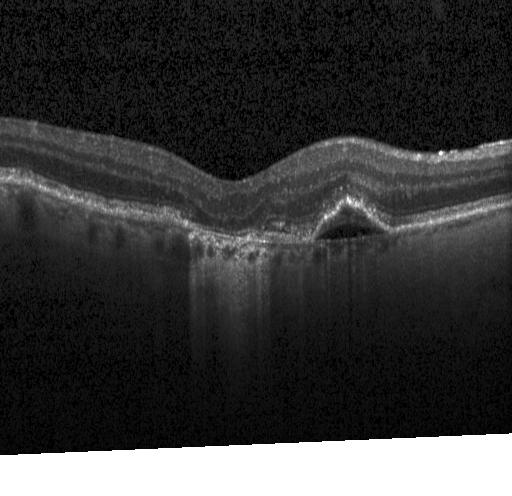

Optical coherence tomography scan. Acquired on a Heidelberg Spectralis.
Choroidal neovascularization (CNV).